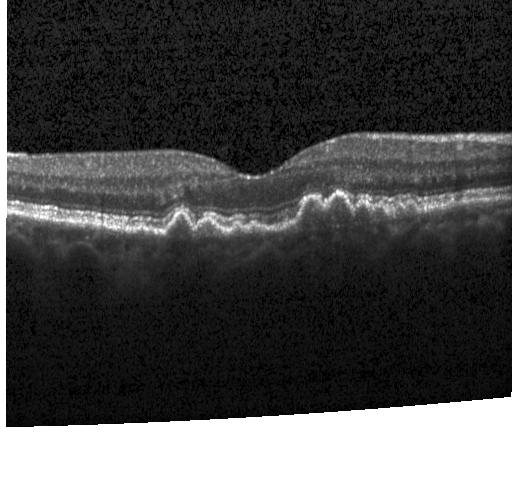
OCT B-scan showing multiple drusen.